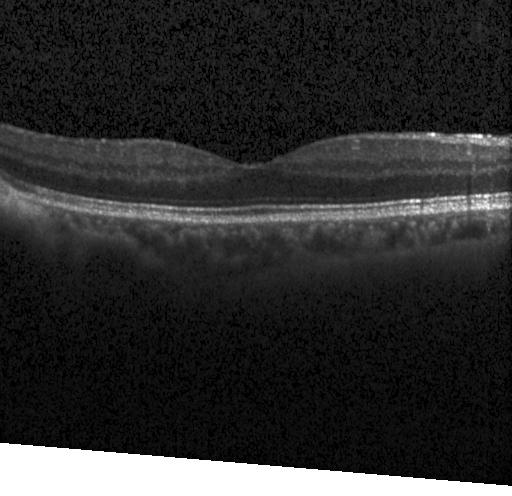 Fovea-centered, Heidelberg Spectralis OCT system, optical coherence tomography scan, SD-OCT. Diagnosis: no evidence of choroidal neovascularization, diabetic macular edema, or drusen.